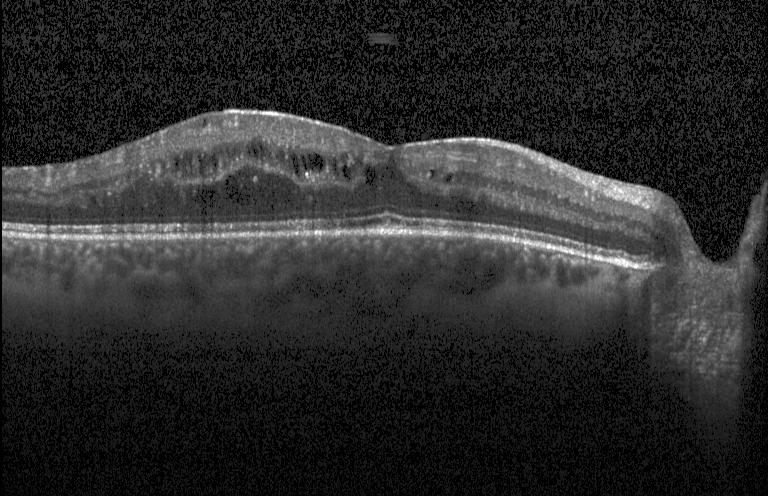
Heidelberg Spectralis OCT system; retinal OCT B-scan — Dx: diabetic macular edema (DME).